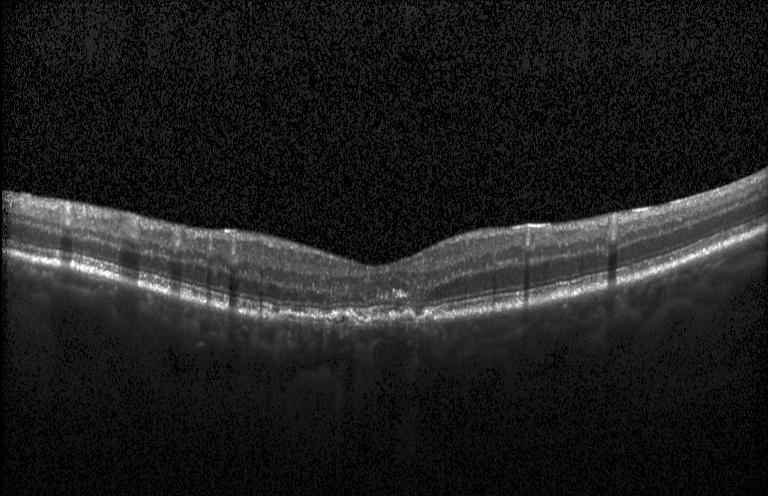
OCT B-scan — Finding: a choroidal neovascular membrane.